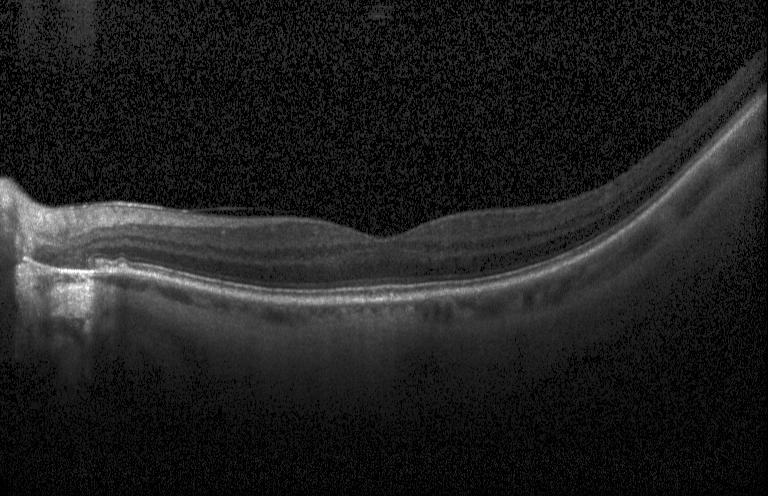 Optical coherence tomography scan; acquired on a Heidelberg Spectralis; centered on the fovea. Impression: no evidence of choroidal neovascularization, diabetic macular edema, or drusen.